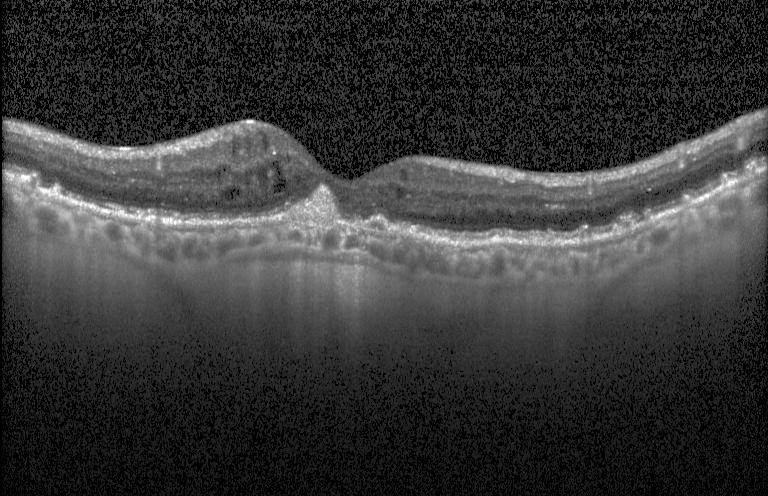

Optical coherence tomography scan.
Diagnosis: a choroidal neovascular membrane.